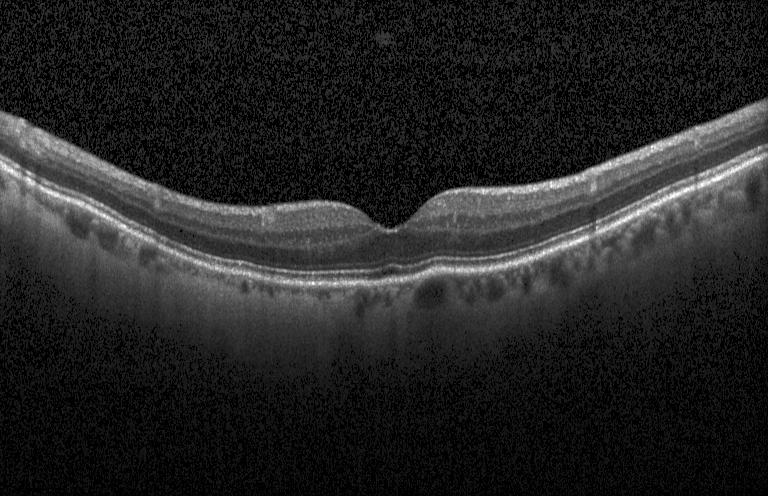

Retinal OCT B-scan. Impression: neither choroidal neovascularization, diabetic macular edema, nor drusen.